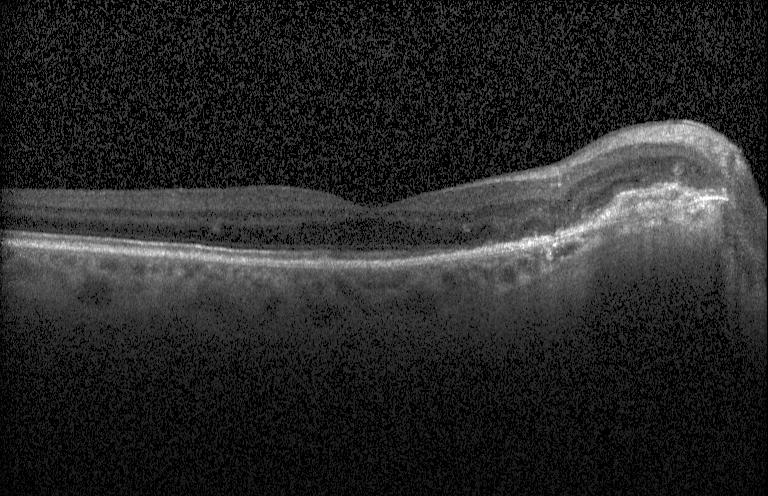
OCT line scan
The scan shows a choroidal neovascular membrane.